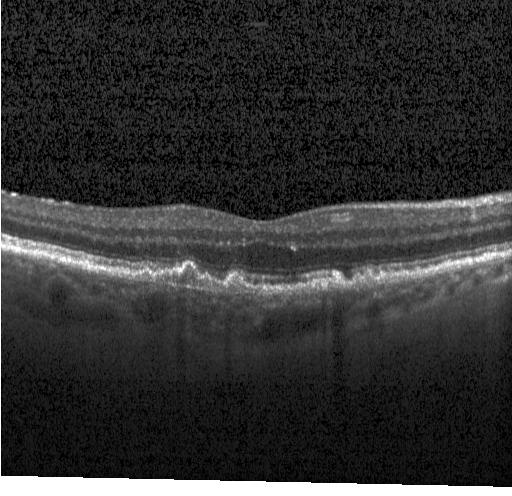 Optical coherence tomography scan · spectral-domain OCT · Heidelberg Spectralis OCT system.
OCT finding: a choroidal neovascular membrane.